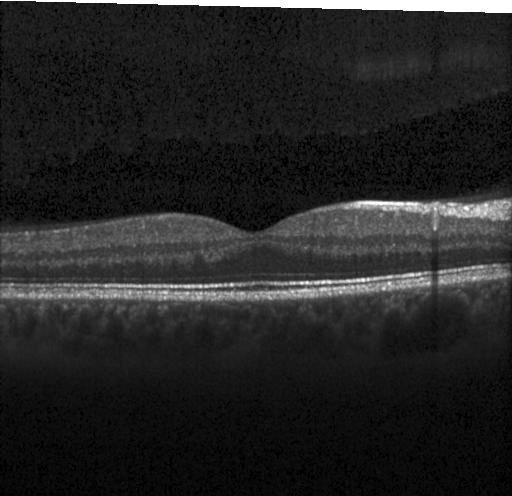

Impression: no choroidal neovascularization, diabetic macular edema, or drusen.